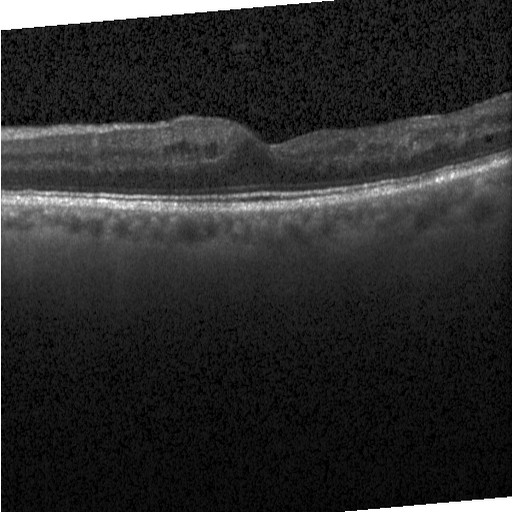
Retinal OCT cross-section showing DME.